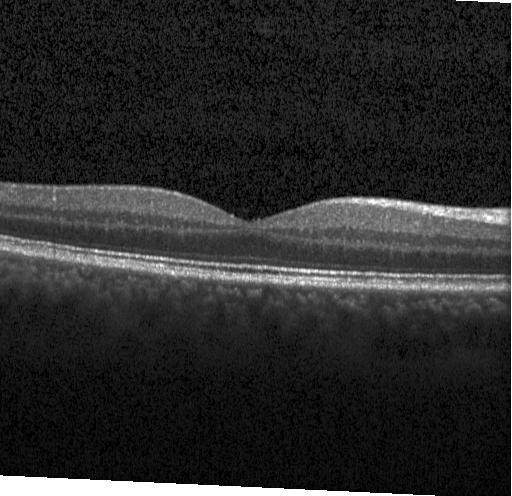 Impression: neither choroidal neovascularization, diabetic macular edema, nor drusen.